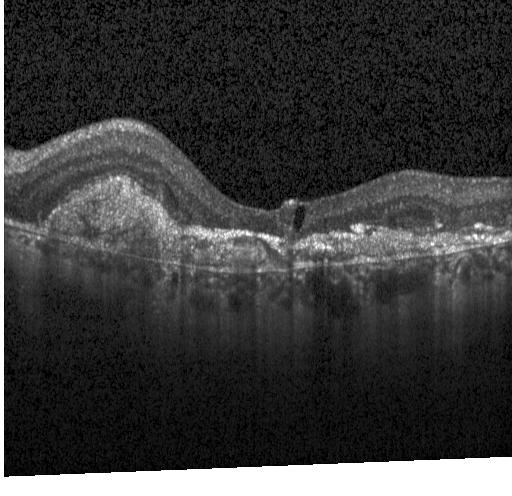 OCT B-scan
OCT finding: a choroidal neovascular membrane.